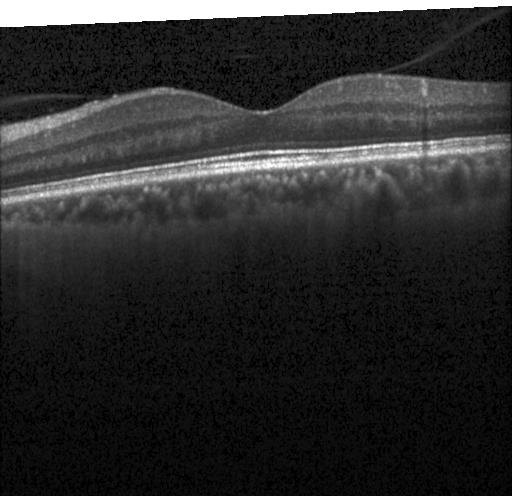
Optical coherence tomography scan · instrument: Heidelberg Spectralis · through the macula · spectral-domain optical coherence tomography — Dx: no evidence of choroidal neovascularization, diabetic macular edema, or drusen.